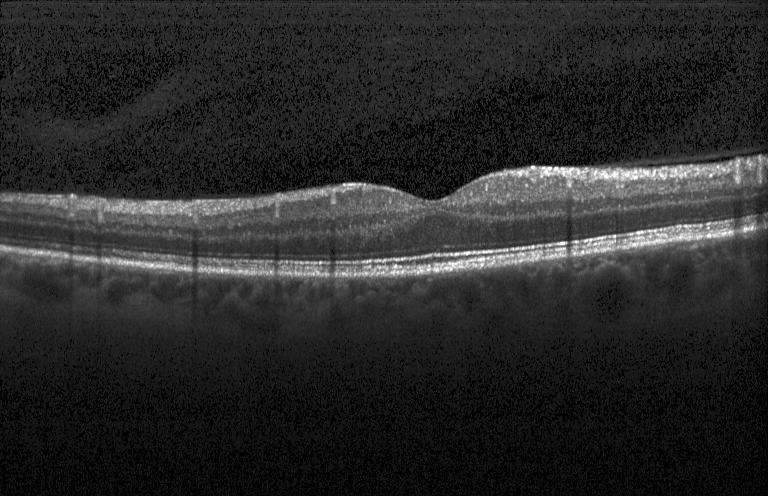
Macular OCT: no CNV, DME, or drusen.